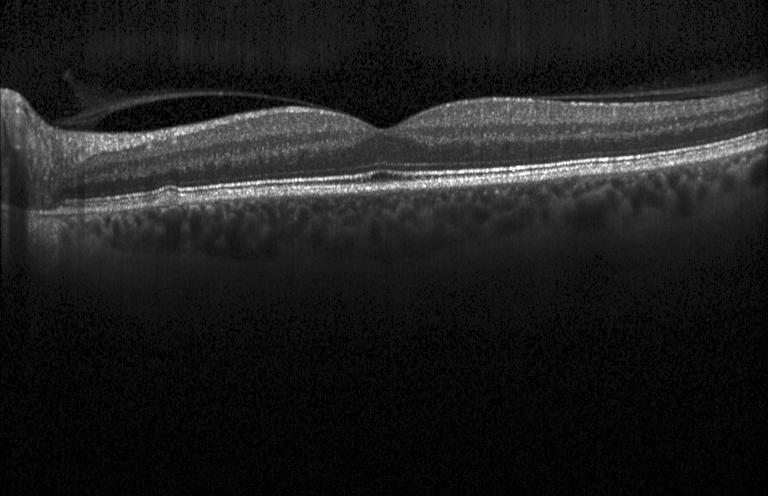

OCT line scan · macular scan · instrument: Heidelberg Spectralis
Finding: neither choroidal neovascularization, diabetic macular edema, nor drusen.